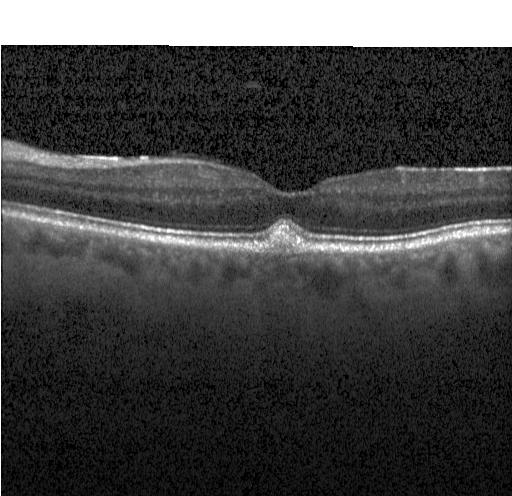 Macular OCT demonstrating multiple drusen.